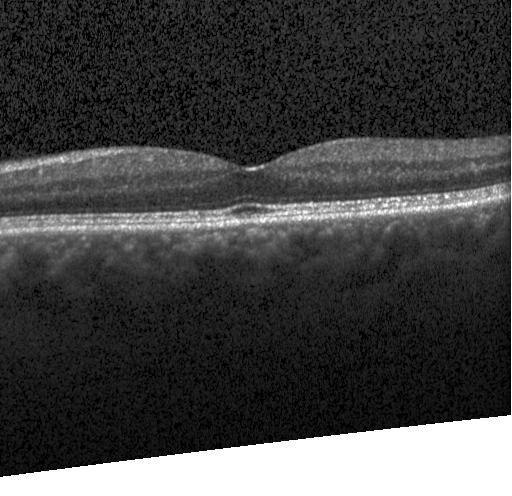
SD-OCT; centered on the fovea; retinal OCT cross-section; Heidelberg Spectralis OCT system
Diagnosis: no evidence of choroidal neovascularization, diabetic macular edema, or drusen.